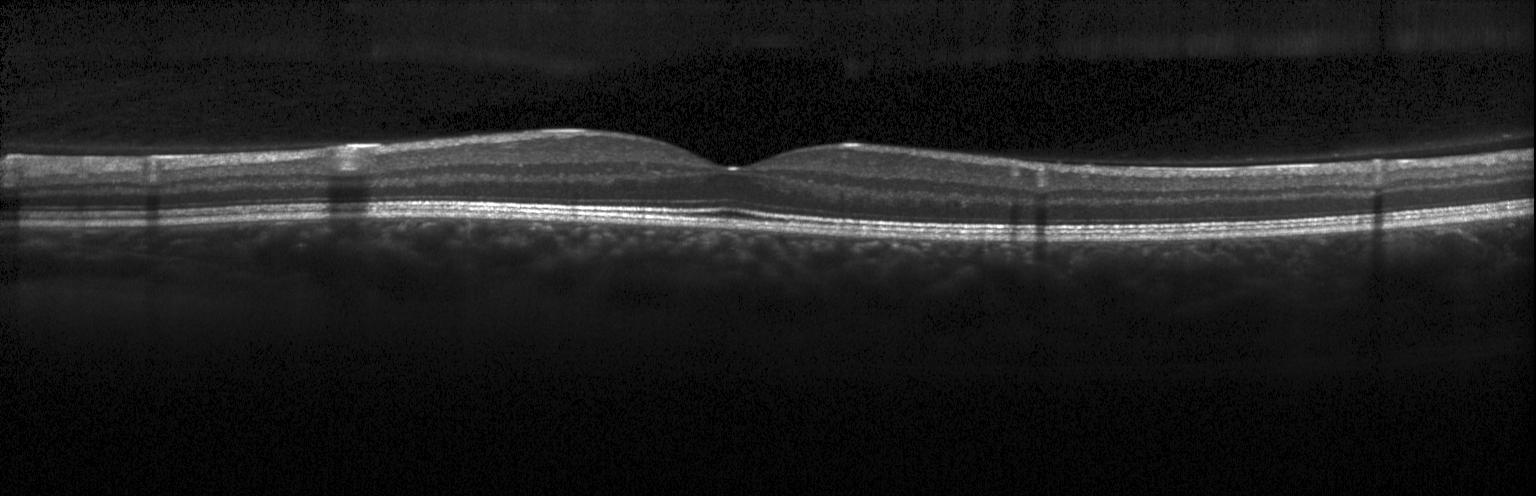 Retinal OCT cross-section
Assessment: no CNV, DME, or drusen.